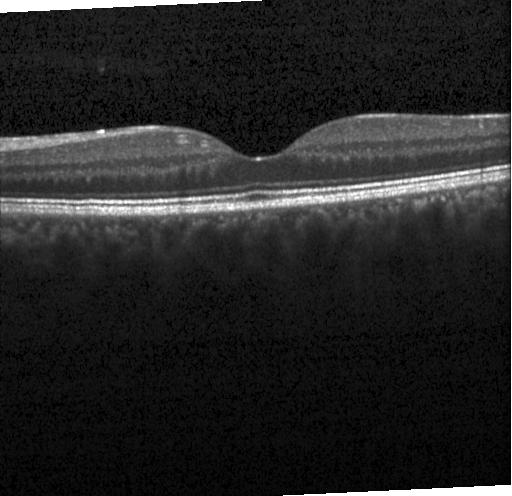
OCT line scan.
Macular OCT: no CNV, no DME, and no drusen.